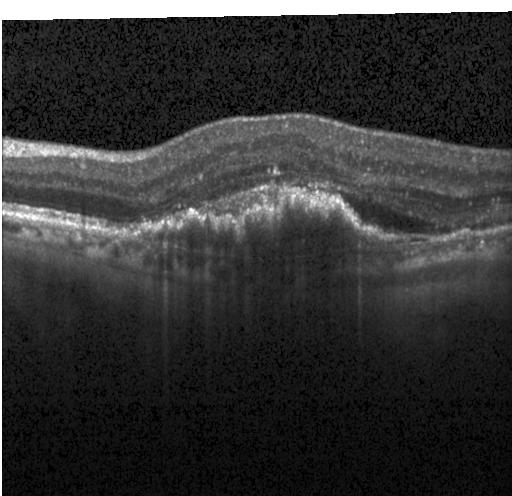
Retinal OCT cross-section. Finding: CNV.